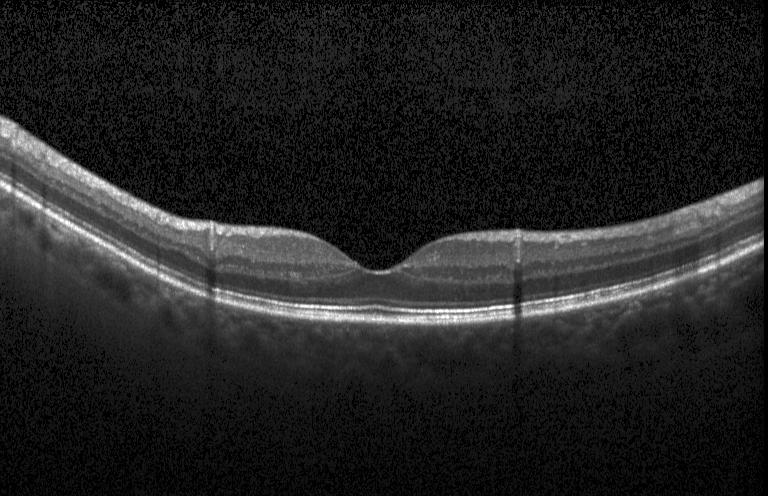
Retinal OCT B-scan — Diagnosis: no CNV, no DME, and no drusen.